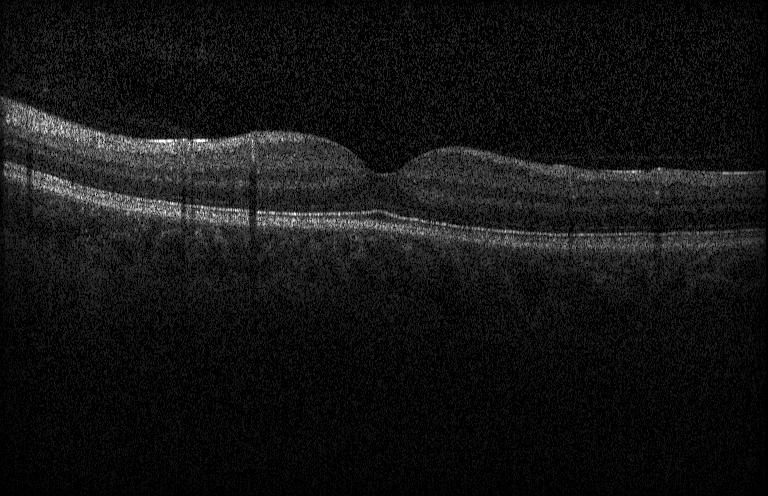
Retinal OCT B-scan, through the macula — OCT finding: no choroidal neovascularization, diabetic macular edema, or drusen.